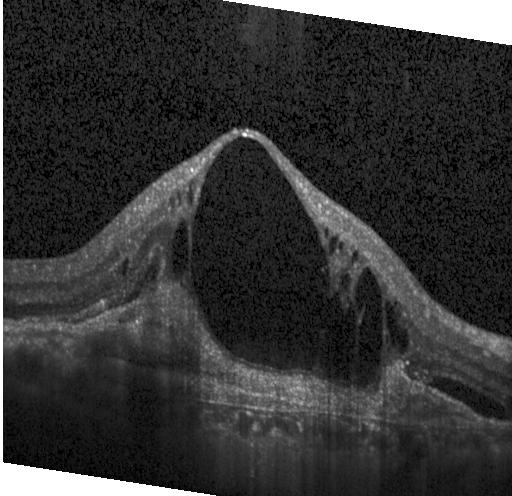

A choroidal neovascular membrane.